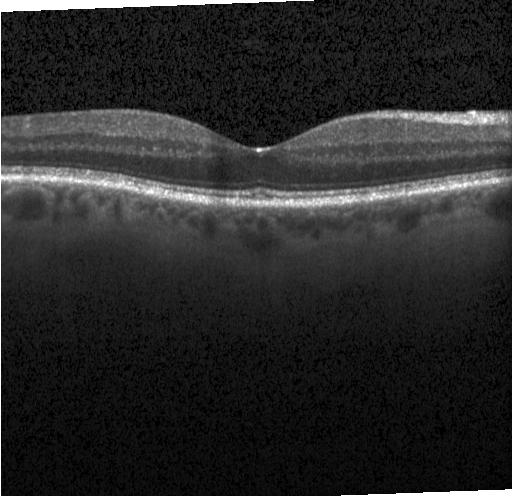 Macular OCT: neither choroidal neovascularization, diabetic macular edema, nor drusen.